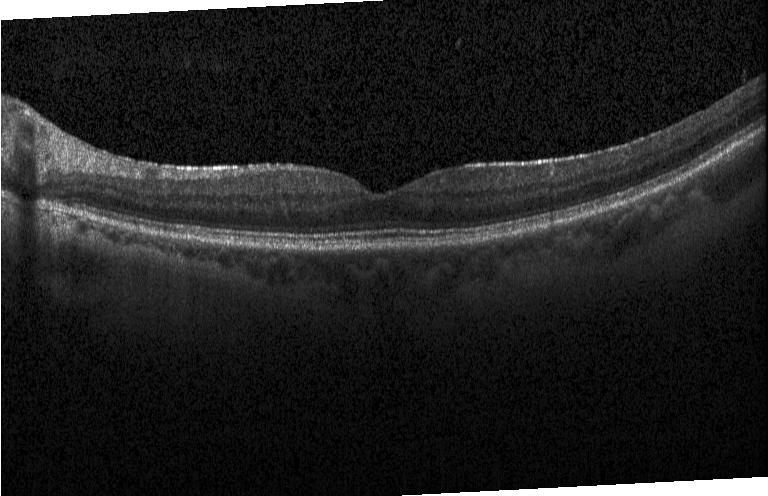

Heidelberg Spectralis OCT system; through the macula; optical coherence tomography scan — Impression: no choroidal neovascularization, diabetic macular edema, or drusen.